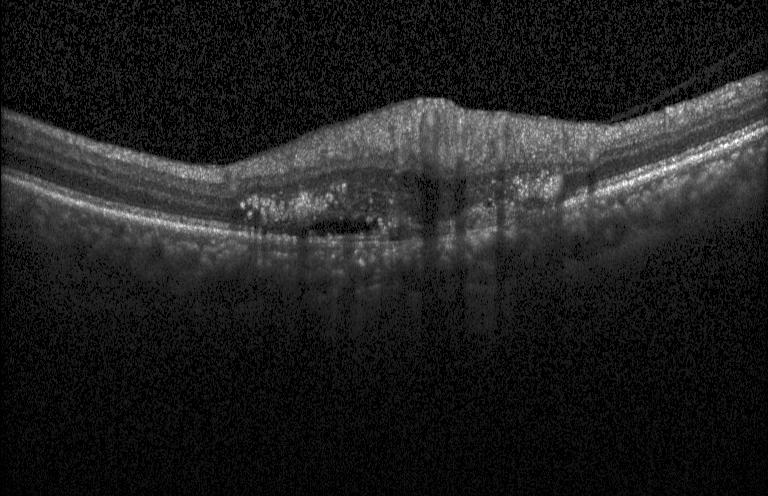
Horizontal scan through the fovea · spectral-domain OCT · optical coherence tomography scan · instrument: Heidelberg Spectralis.
A choroidal neovascular membrane.